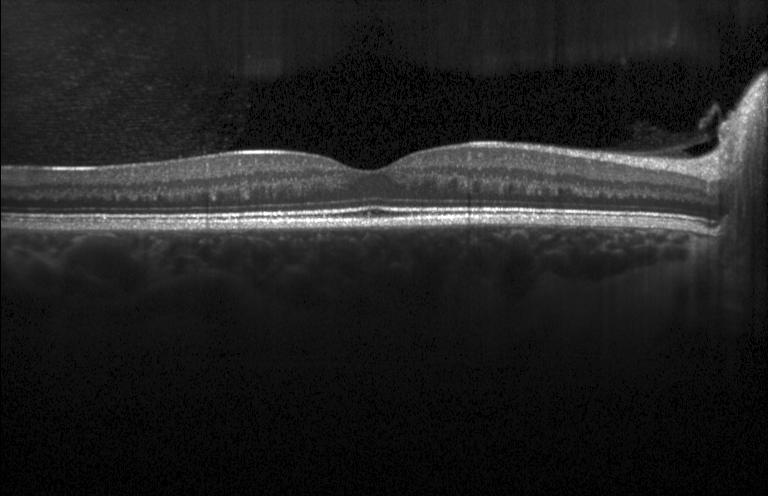 Macular scan, acquired on a Heidelberg Spectralis, retinal OCT cross-section, SD-OCT — Impression: neither CNV, DME, nor drusen.